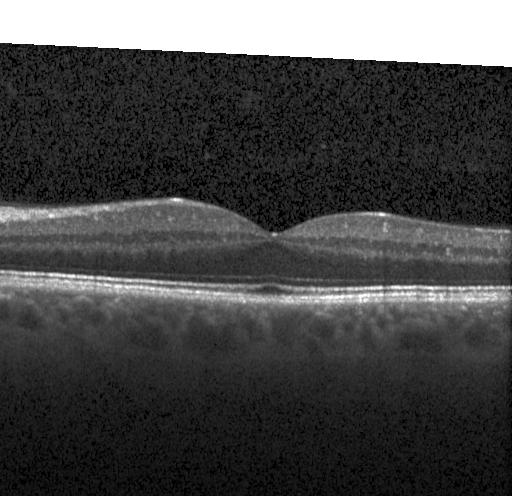

Dx: no CNV, no DME, and no drusen.